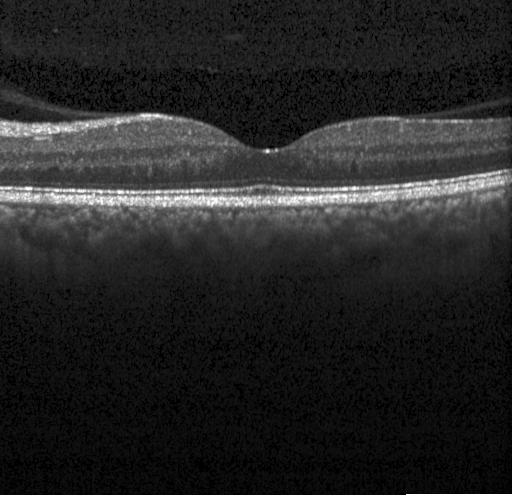
OCT B-scan showing no CNV, no DME, and no drusen.